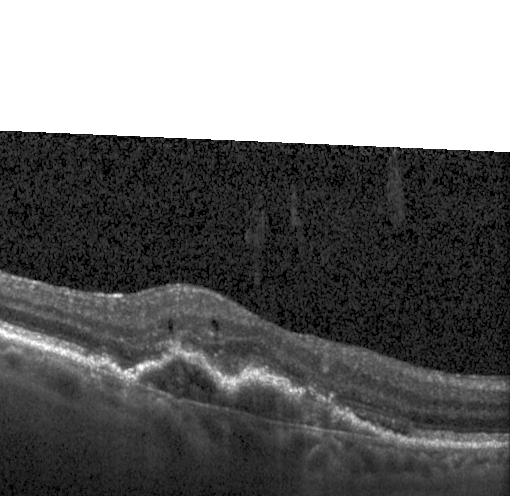 Dx: a choroidal neovascular membrane.